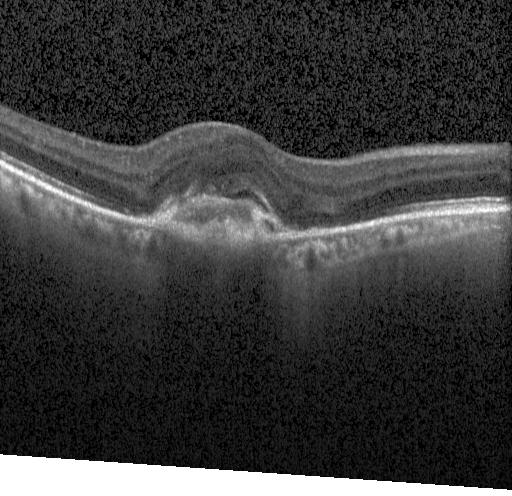 Heidelberg Spectralis OCT system; optical coherence tomography B-scan.
Macular OCT: CNV.